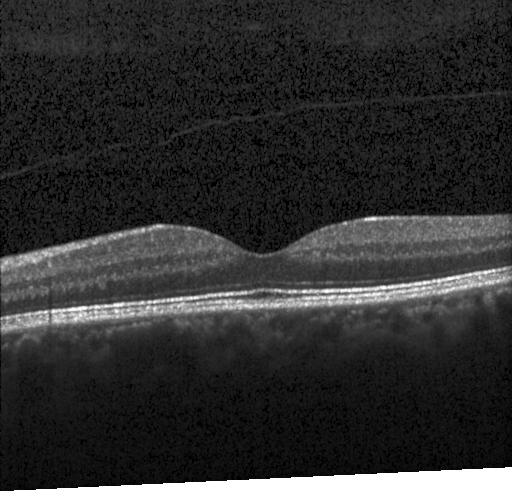

SD-OCT; retinal OCT B-scan — Macular OCT: no choroidal neovascularization, no diabetic macular edema, and no drusen.